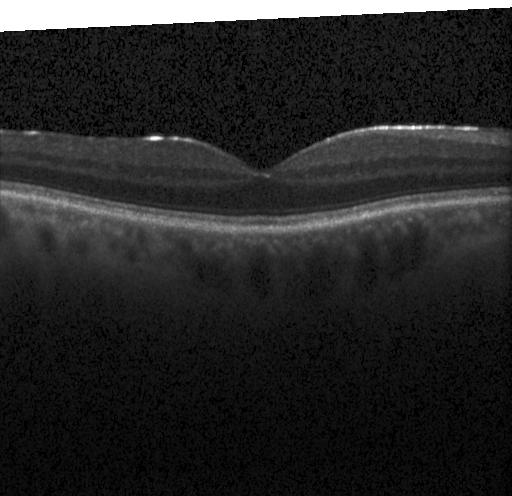

Impression: no evidence of choroidal neovascularization, diabetic macular edema, or drusen.